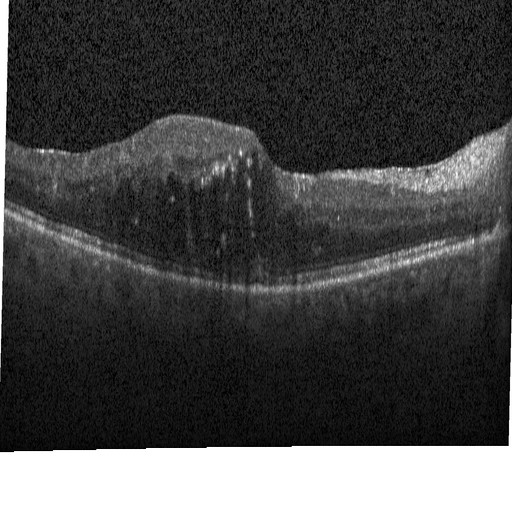

Impression: diabetic macular edema.